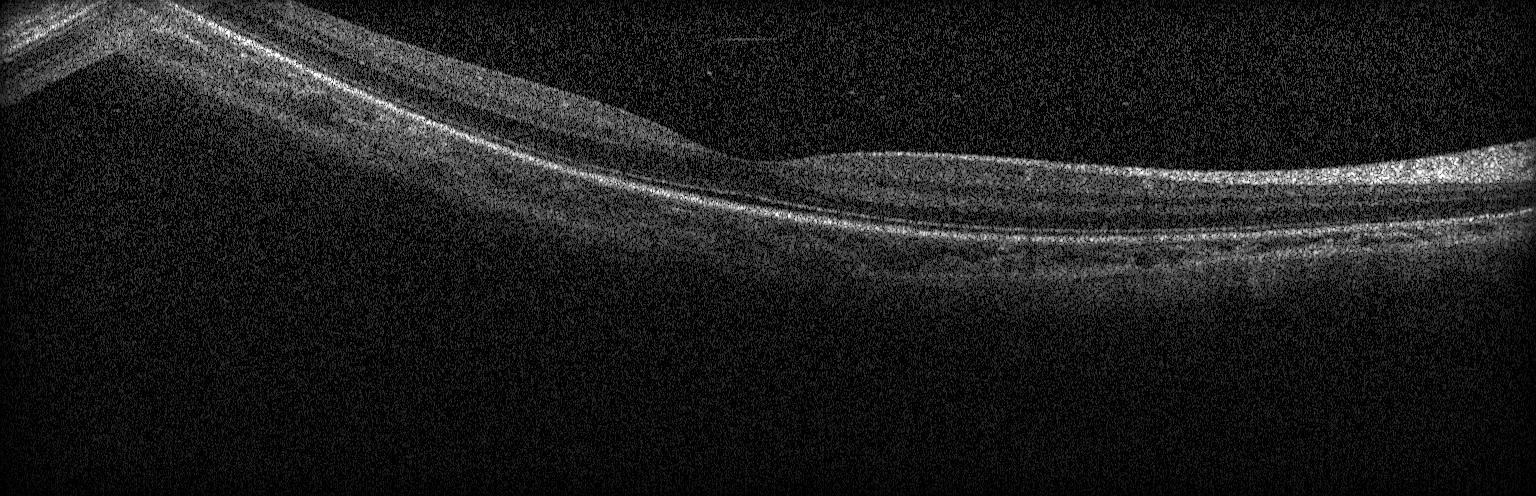 Macular OCT demonstrating no choroidal neovascularization, diabetic macular edema, or drusen.